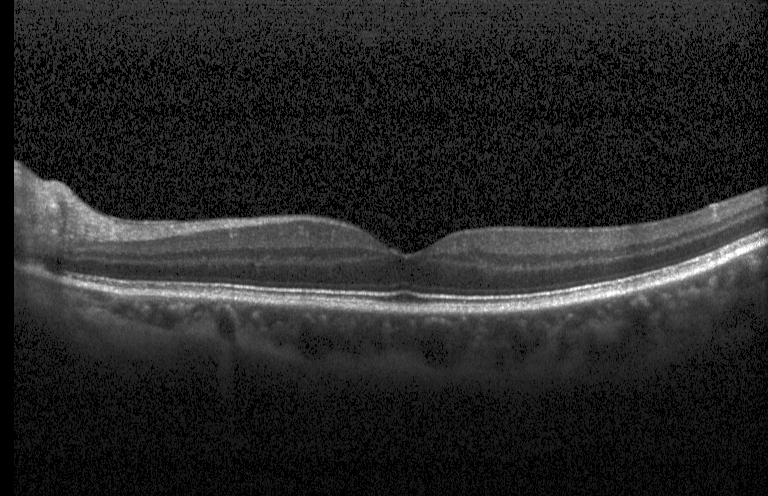
Diagnosis: no choroidal neovascularization, no diabetic macular edema, and no drusen.